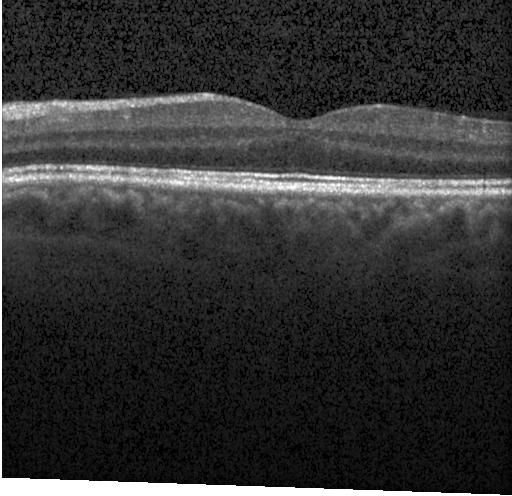
Dx: no evidence of choroidal neovascularization, diabetic macular edema, or drusen.